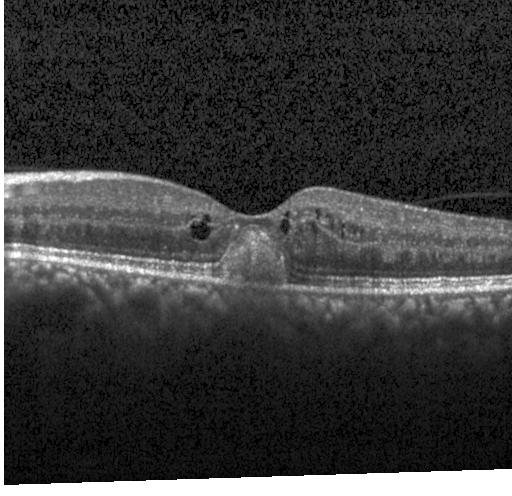
OCT B-scan showing a choroidal neovascular membrane.